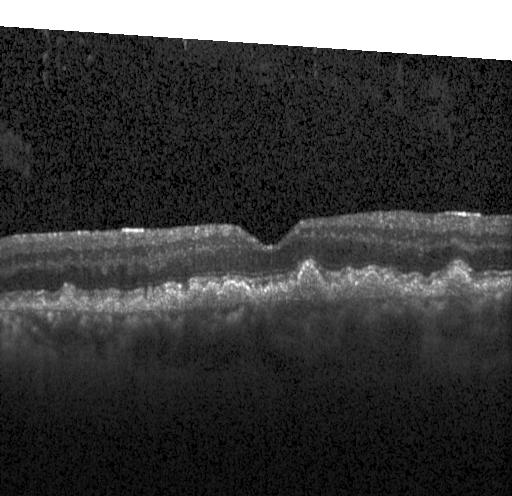
Horizontal scan through the fovea; SD-OCT; retinal OCT cross-section — Dx: a choroidal neovascular membrane.